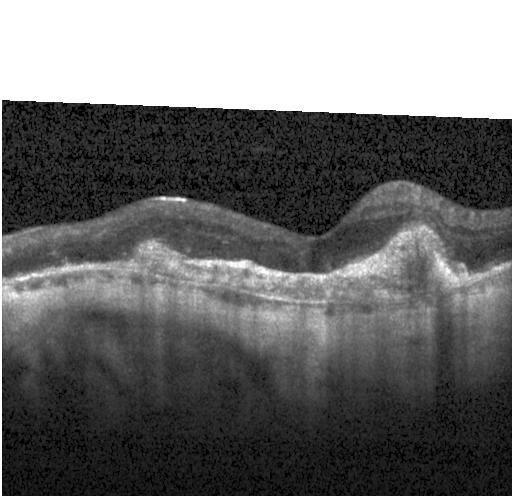

Optical coherence tomography scan
OCT finding: a choroidal neovascular membrane.